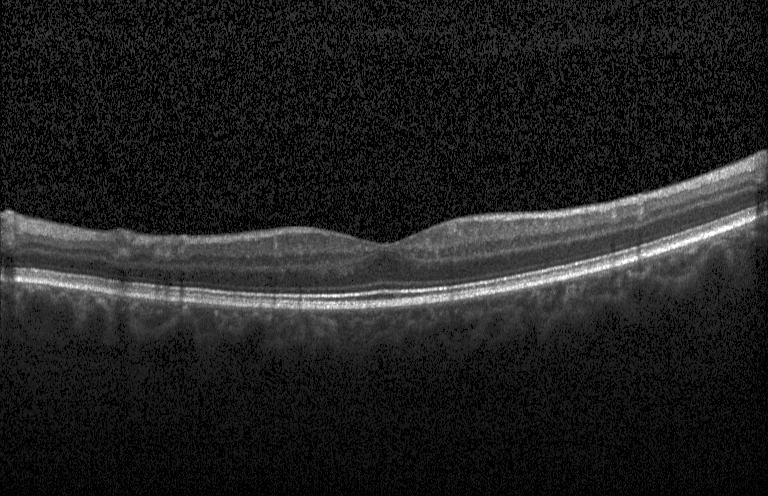

Instrument: Heidelberg Spectralis · OCT B-scan · through the macula · spectral-domain optical coherence tomography
This B-scan demonstrates neither choroidal neovascularization, diabetic macular edema, nor drusen.